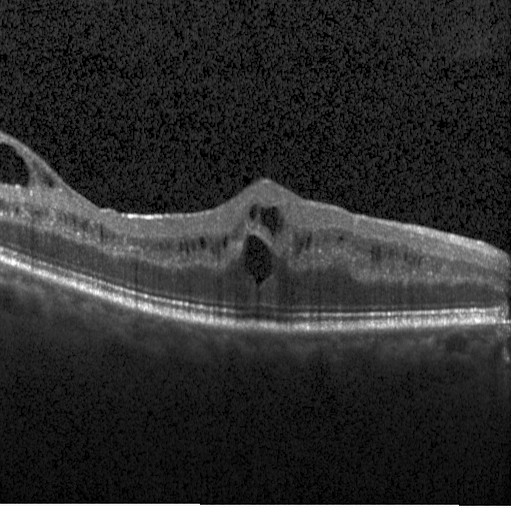
Impression: DME.